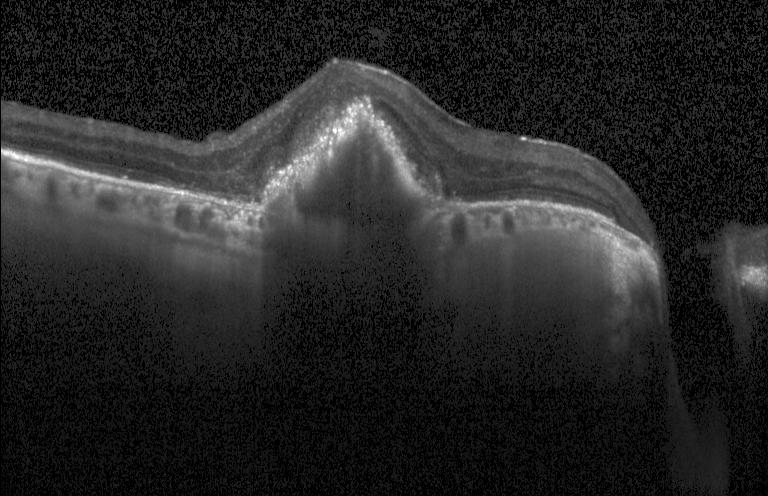
OCT B-scan, spectral-domain optical coherence tomography, centered on the fovea — Choroidal neovascularization (CNV).